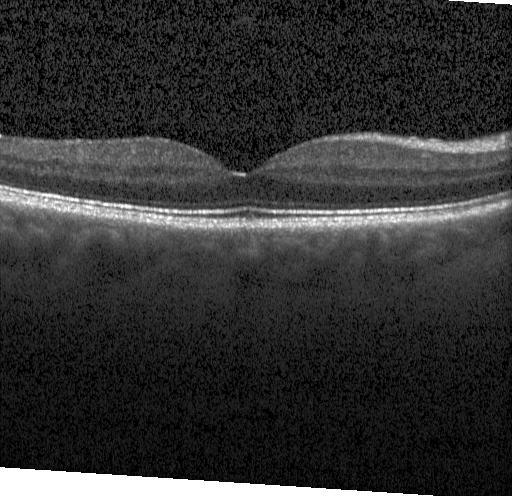 Spectral-domain OCT · retinal OCT cross-section · horizontal scan through the fovea — Impression: no evidence of choroidal neovascularization, diabetic macular edema, or drusen.